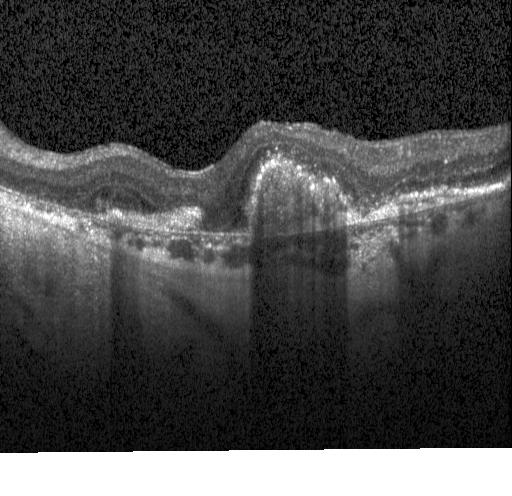
Optical coherence tomography B-scan. Finding: a choroidal neovascular membrane.